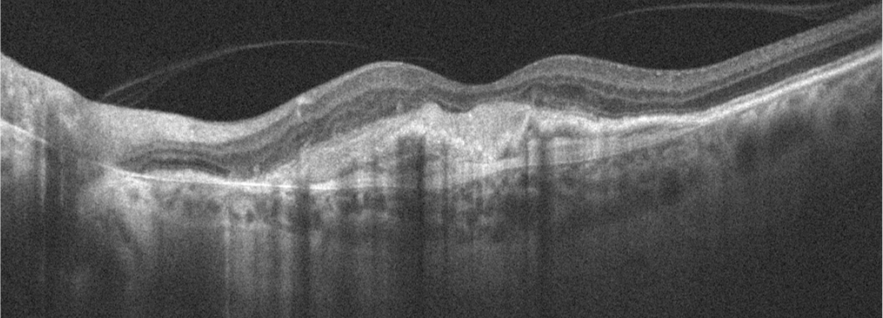

Fovea-centered · retinal OCT B-scan — OCT finding: AMD.